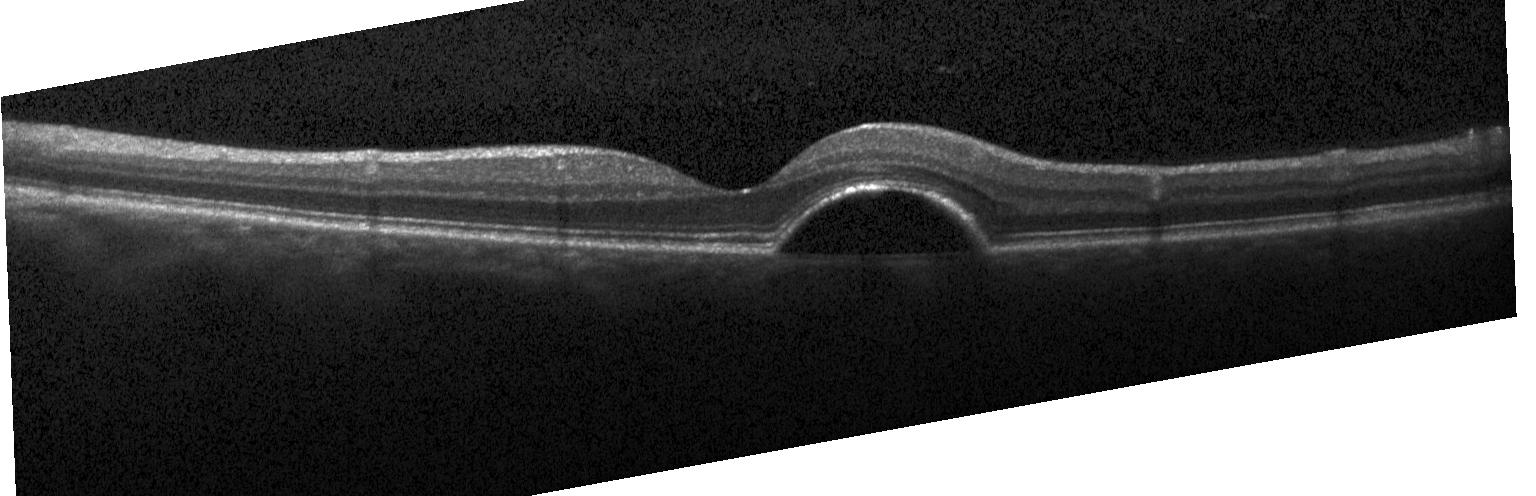 Retinal OCT B-scan. Macular OCT: CNV.